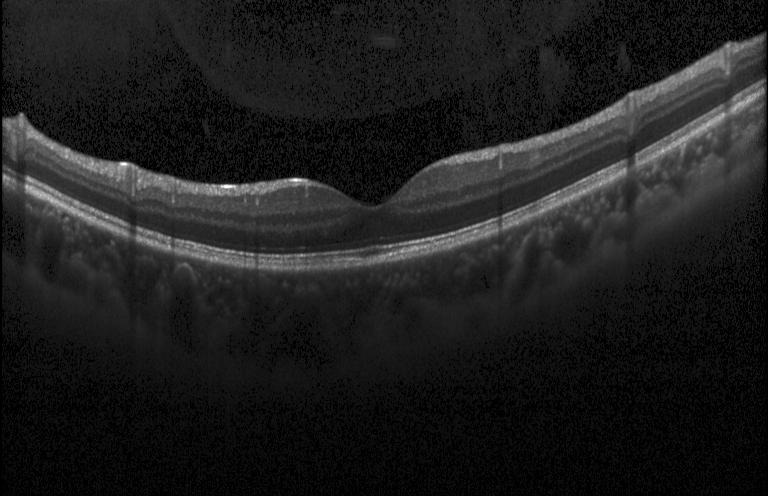 Macular OCT: no CNV, no DME, and no drusen.